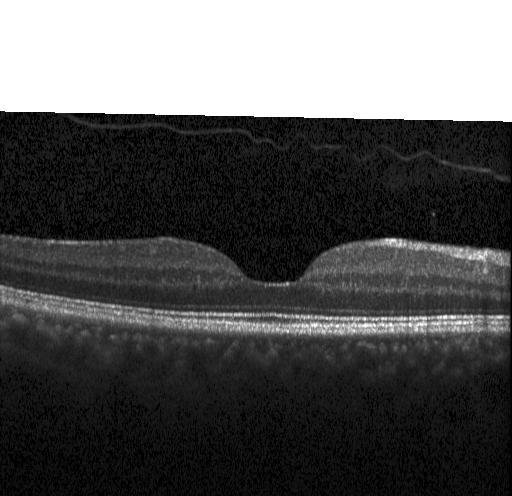 Diagnosis: no CNV, DME, or drusen.